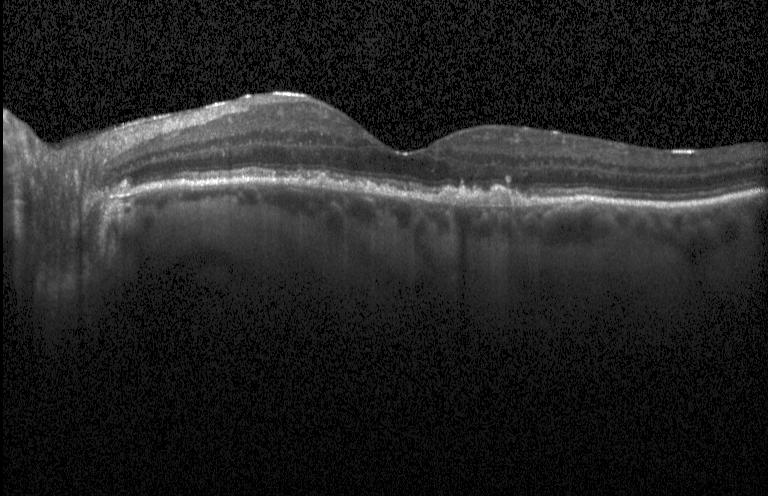

Heidelberg Spectralis · optical coherence tomography scan · spectral-domain OCT.
Assessment: drusen.